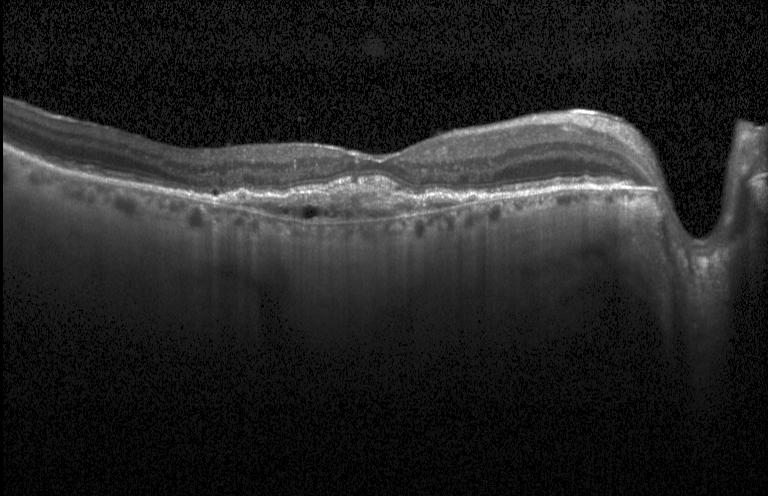
Retinal OCT cross-section.
Finding: a choroidal neovascular membrane.